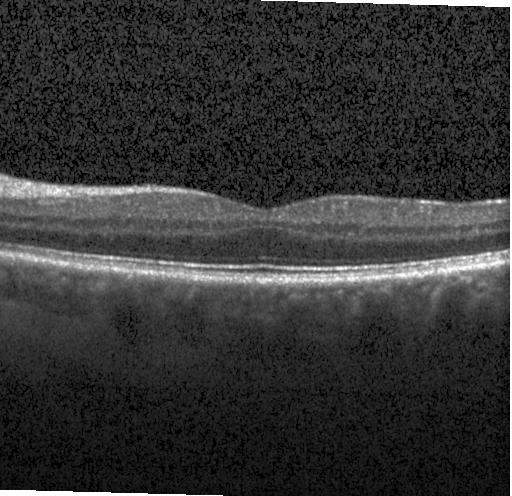

Assessment: no choroidal neovascularization, diabetic macular edema, or drusen.